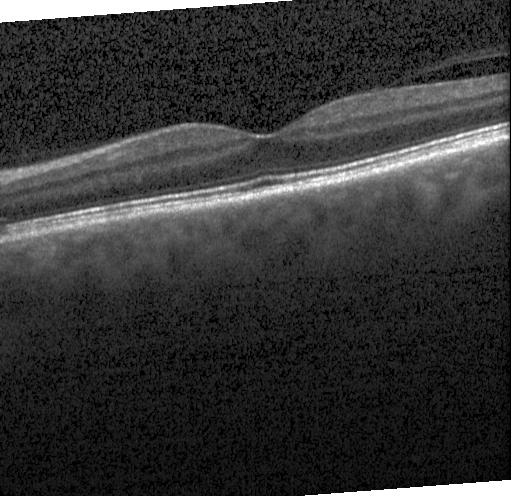

Retinal OCT cross-section
Dx: no evidence of choroidal neovascularization, diabetic macular edema, or drusen.